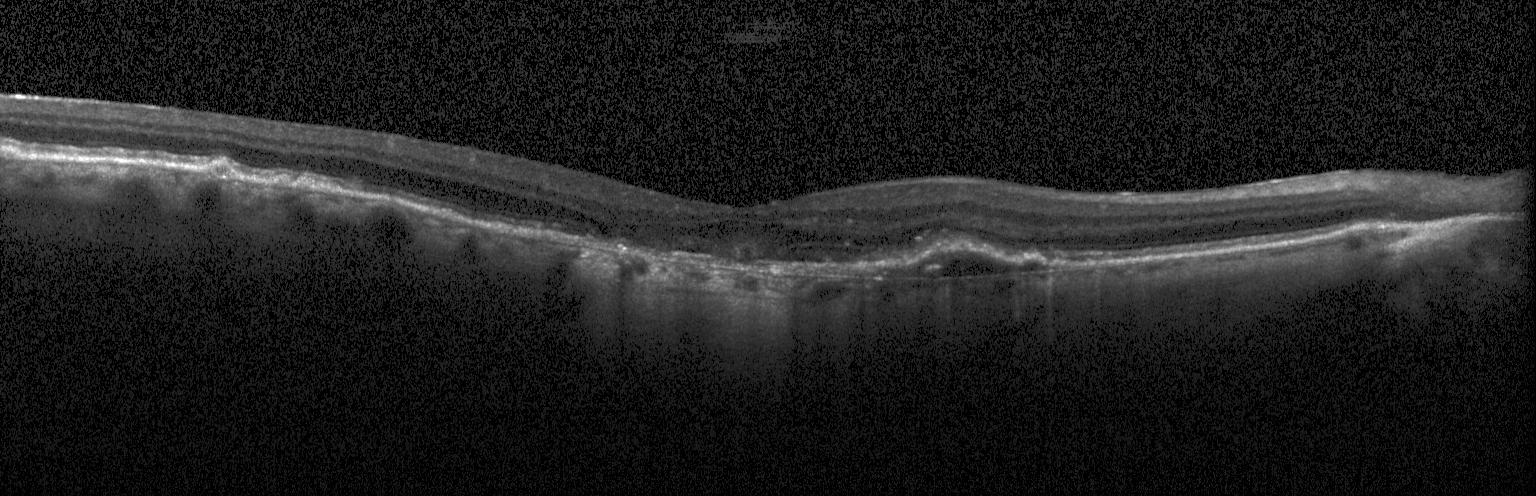 OCT scan showing a choroidal neovascular membrane.